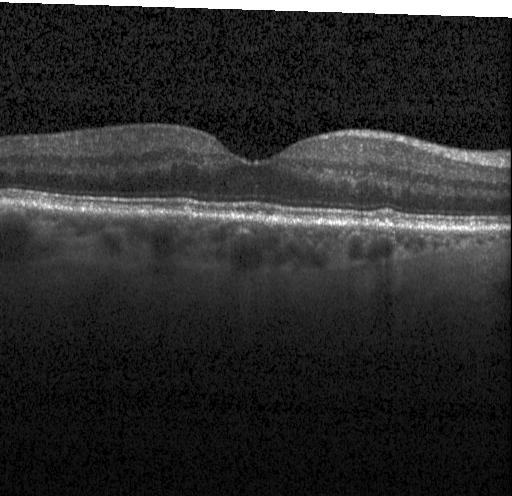
OCT B-scan. Heidelberg Spectralis OCT system. Diagnosis: neither choroidal neovascularization, diabetic macular edema, nor drusen.